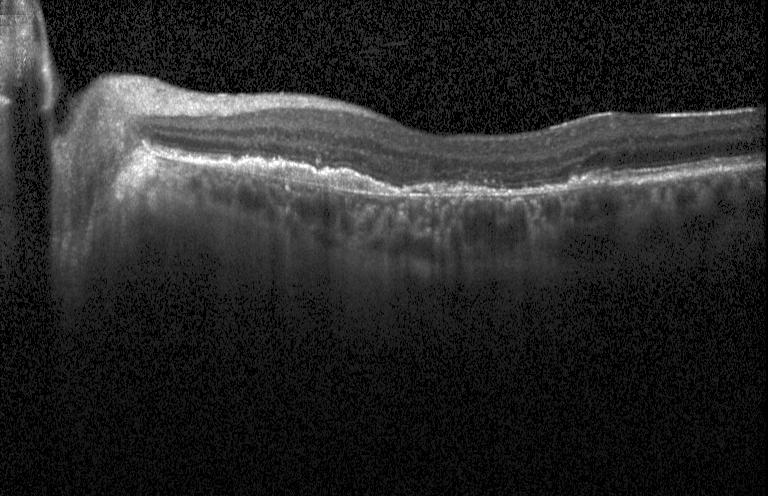 OCT scan showing a choroidal neovascular membrane.